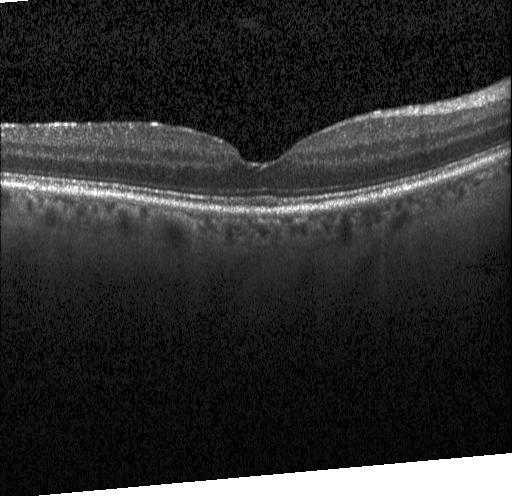 Spectral-domain OCT. Retinal OCT cross-section. Horizontal scan through the fovea. Instrument: Heidelberg Spectralis
Finding: no CNV, no DME, and no drusen.